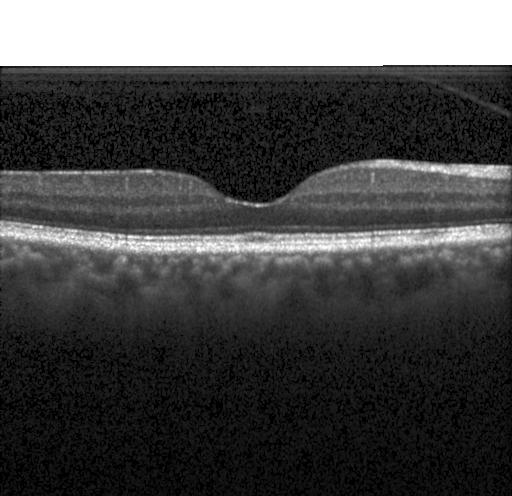
Impression: no CNV, no DME, and no drusen.